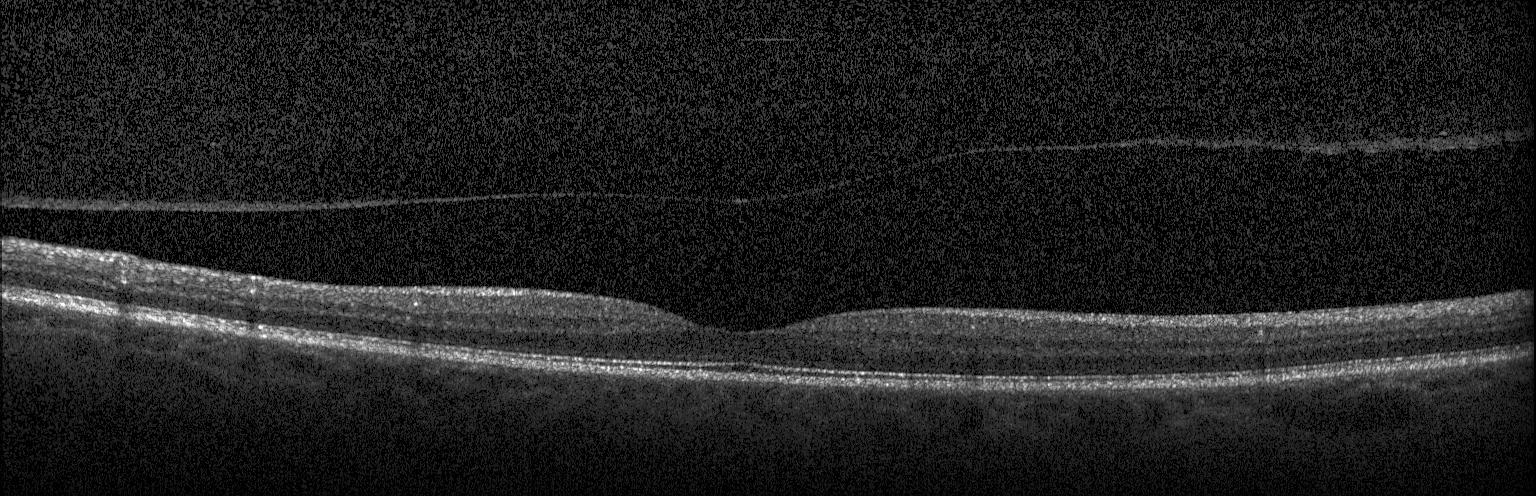 Macular OCT demonstrating no evidence of CNV, DME, or drusen.